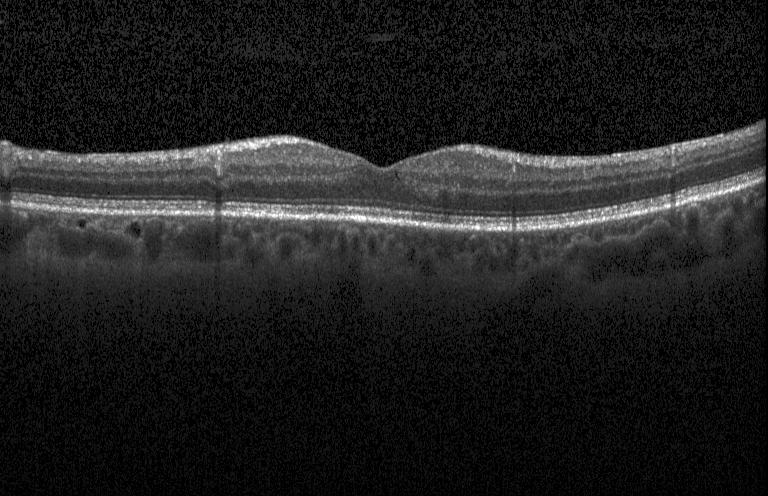

Optical coherence tomography scan, Heidelberg Spectralis, centered on the fovea.
Impression: no choroidal neovascularization, diabetic macular edema, or drusen.